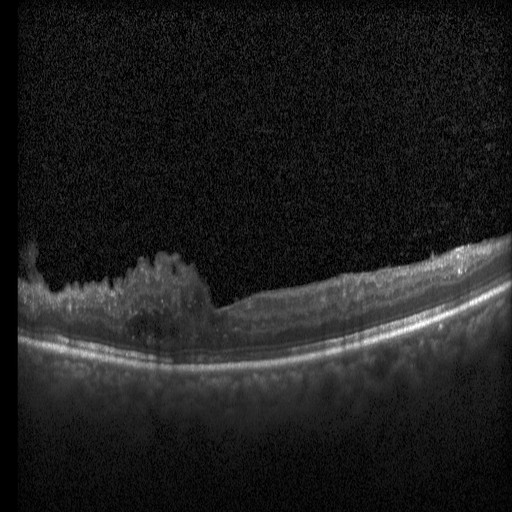

Macular scan. OCT B-scan. Heidelberg Spectralis OCT system. Diagnosis: diabetic macular edema.